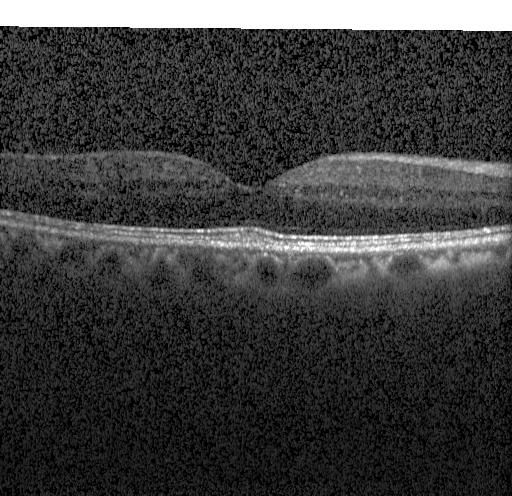

Retinal OCT B-scan. Spectral-domain OCT. Centered on the fovea.
Finding: neither CNV, DME, nor drusen.